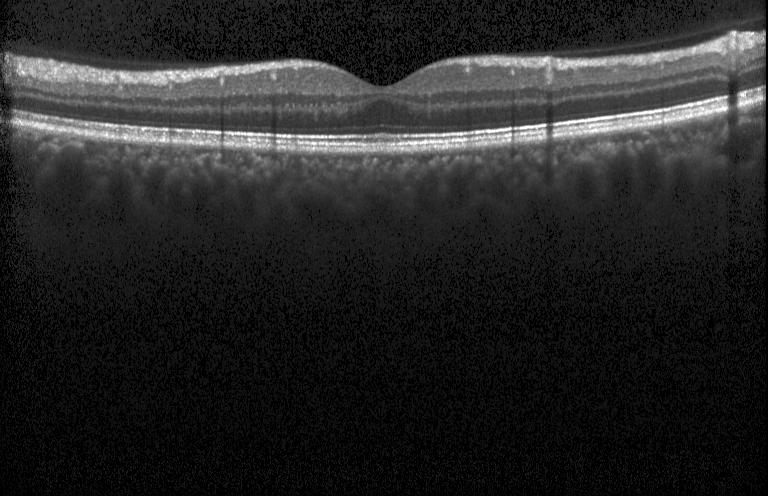
Heidelberg Spectralis. SD-OCT. Macular scan. OCT line scan
Dx: no choroidal neovascularization, diabetic macular edema, or drusen.